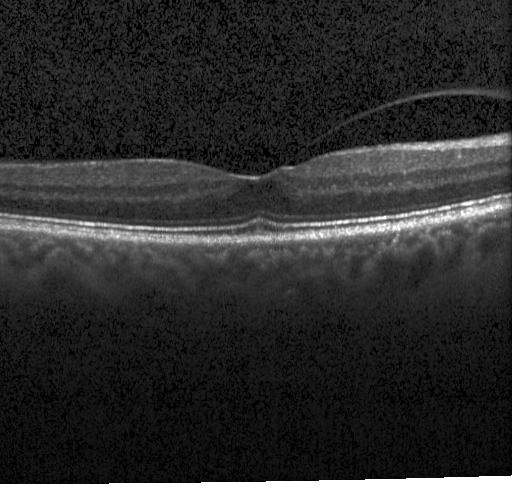
Macular OCT: no evidence of choroidal neovascularization, diabetic macular edema, or drusen.